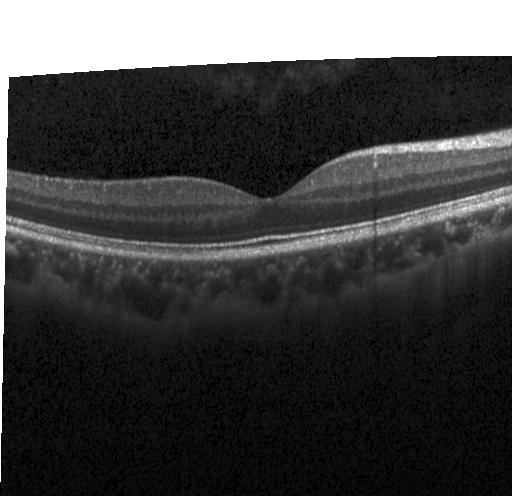 Spectral-domain OCT, acquired on a Heidelberg Spectralis, horizontal scan through the fovea, optical coherence tomography scan. Dx: no CNV, no DME, and no drusen.